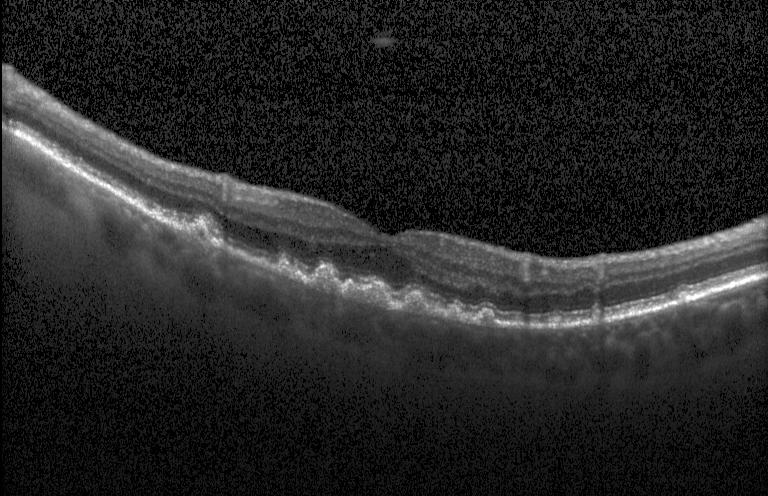 Heidelberg Spectralis; retinal OCT cross-section.
Assessment: multiple drusen.